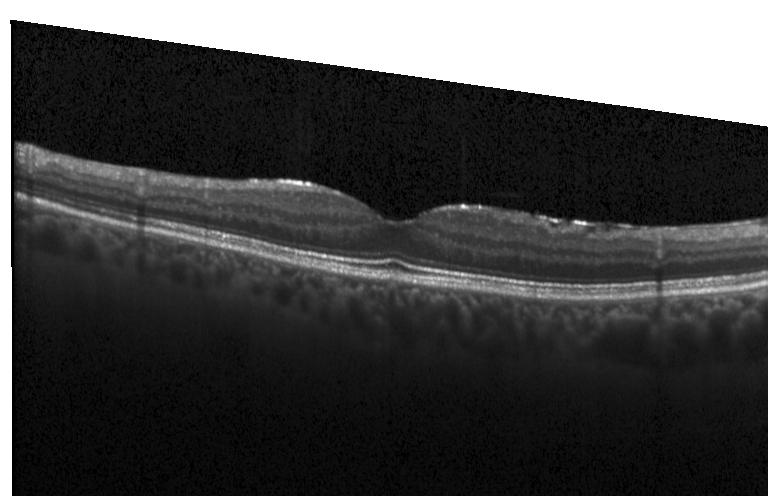

Retinal OCT B-scan — Diagnosis: no choroidal neovascularization, diabetic macular edema, or drusen.